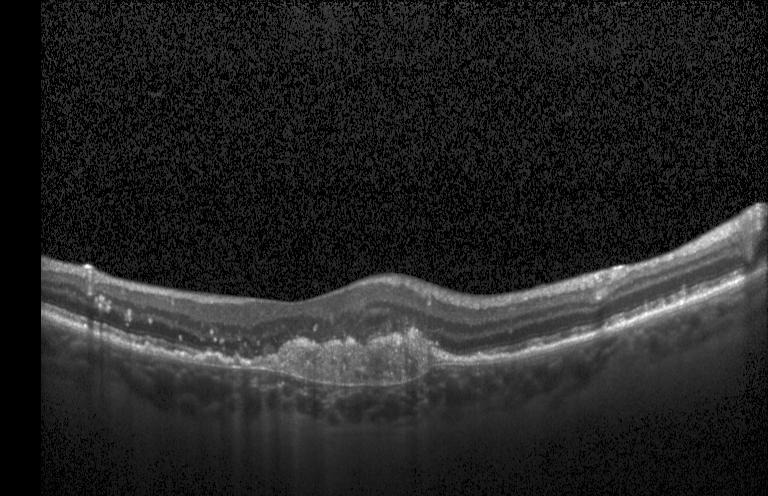
Impression: a choroidal neovascular membrane.